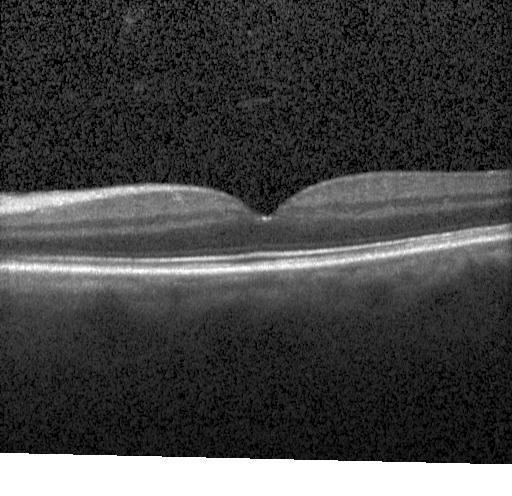

Macular OCT demonstrating neither choroidal neovascularization, diabetic macular edema, nor drusen.